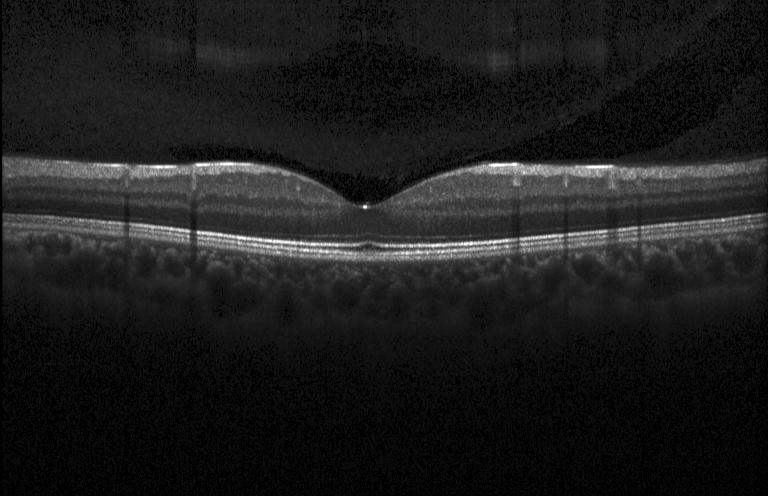
Optical coherence tomography scan.
Diagnosis: no evidence of choroidal neovascularization, diabetic macular edema, or drusen.